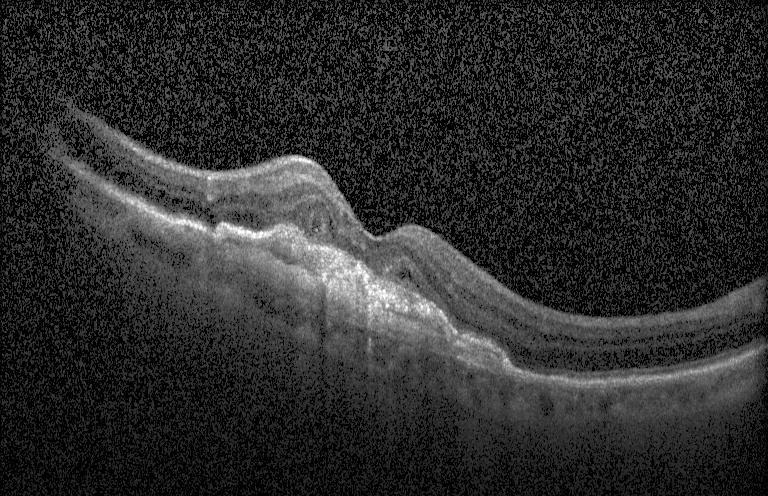 Through the macula, spectral-domain optical coherence tomography, optical coherence tomography B-scan, Heidelberg Spectralis OCT system — This B-scan demonstrates choroidal neovascularization (CNV).